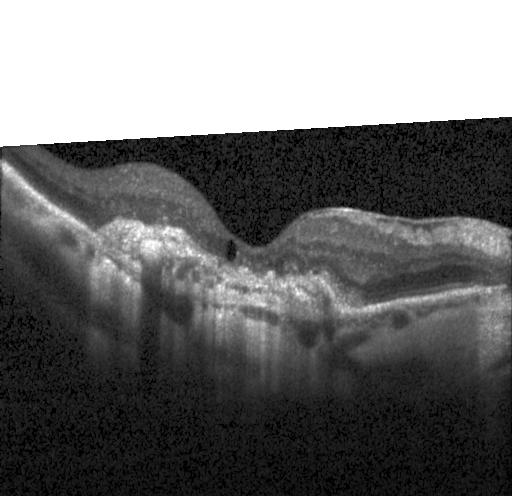

Dx: CNV.